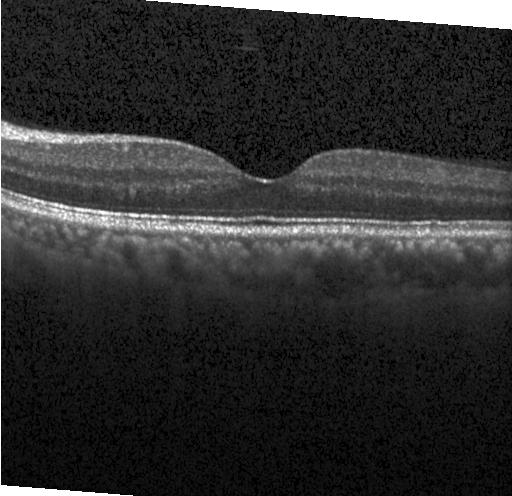
OCT line scan.
Assessment: neither choroidal neovascularization, diabetic macular edema, nor drusen.